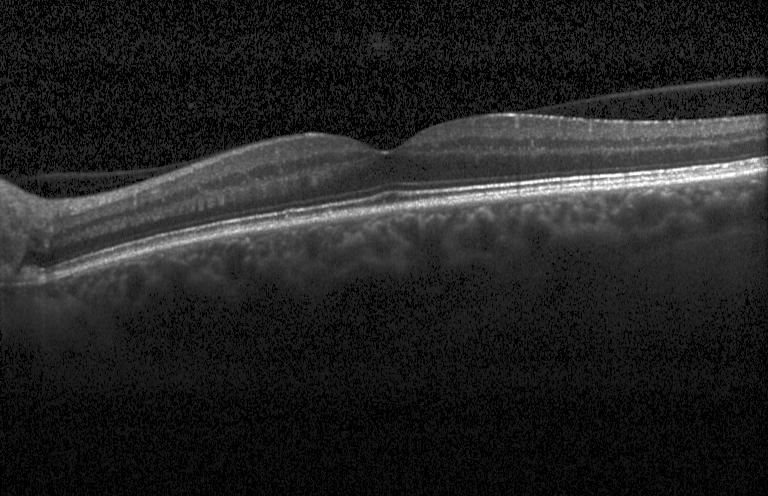

Diagnosis: no choroidal neovascularization, diabetic macular edema, or drusen.